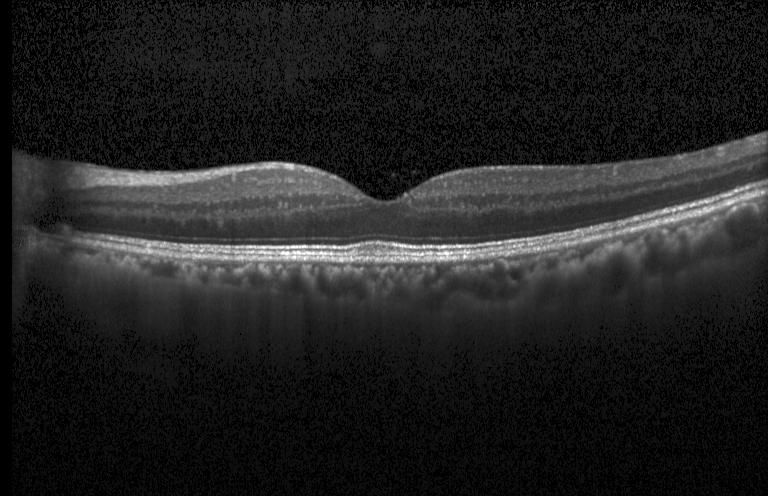
Spectral-domain OCT B-scan: neither choroidal neovascularization, diabetic macular edema, nor drusen.